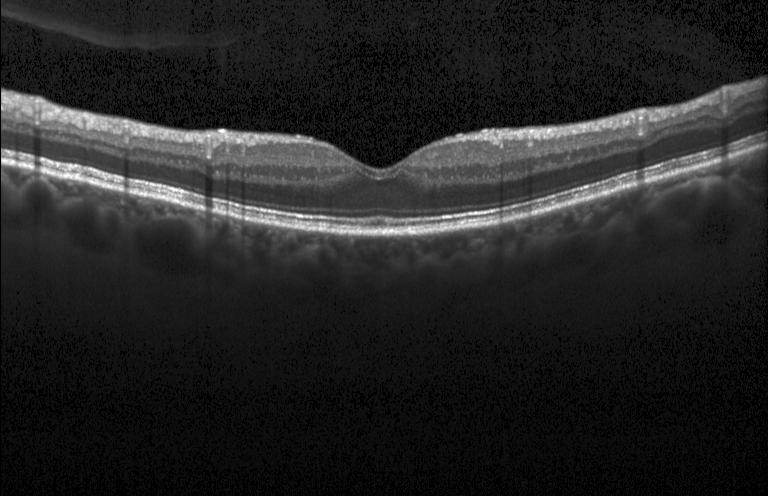 No evidence of choroidal neovascularization, diabetic macular edema, or drusen.